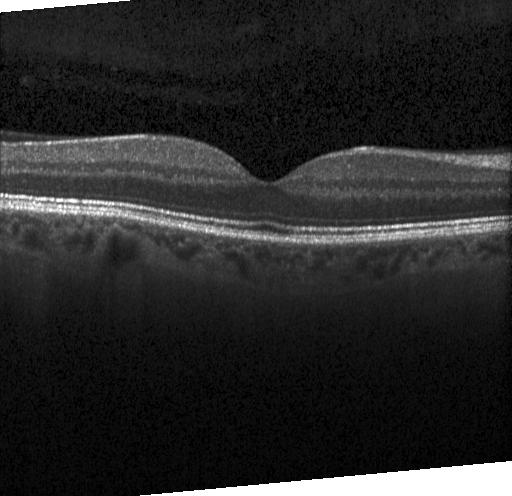 The scan shows no evidence of CNV, DME, or drusen.